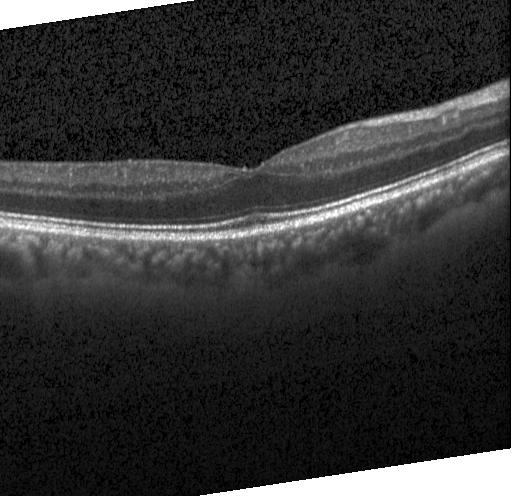

Instrument: Heidelberg Spectralis, macular scan, OCT B-scan.
Finding: neither choroidal neovascularization, diabetic macular edema, nor drusen.